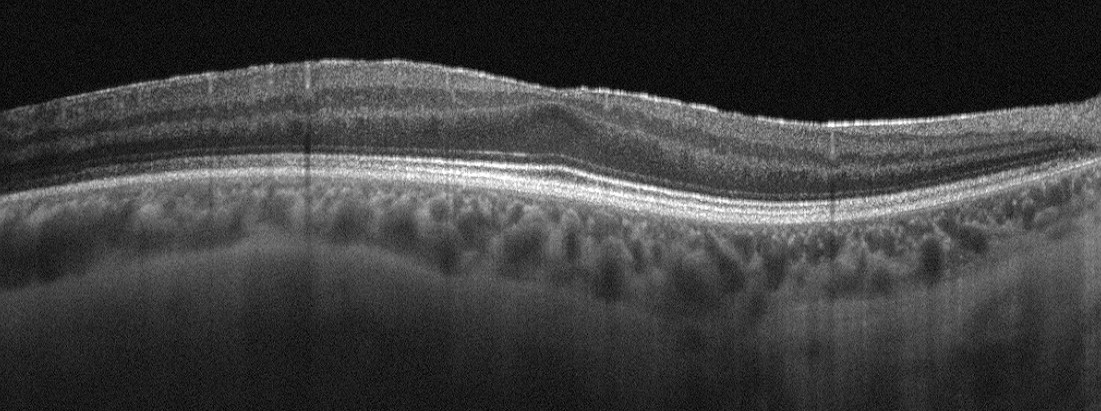 Macular OCT: epiretinal membrane.